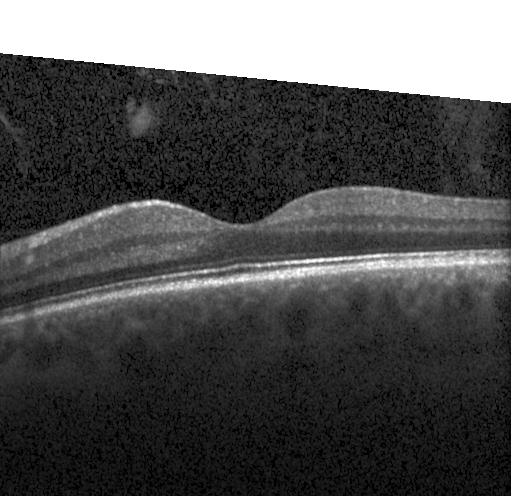

Spectral-domain OCT. Optical coherence tomography scan. Horizontal scan through the fovea
Diagnosis: neither choroidal neovascularization, diabetic macular edema, nor drusen.